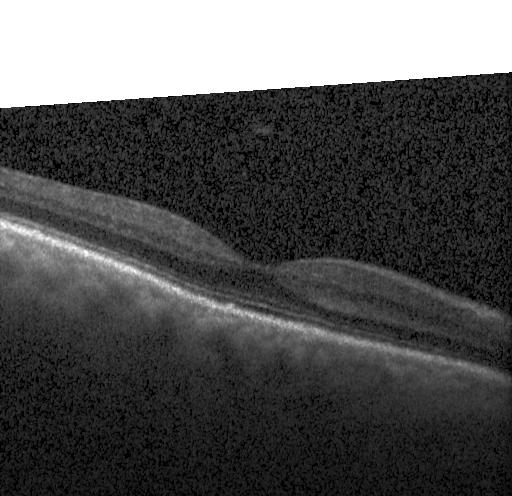 Heidelberg Spectralis · spectral-domain optical coherence tomography · horizontal scan through the fovea · retinal OCT B-scan. Finding: neither choroidal neovascularization, diabetic macular edema, nor drusen.